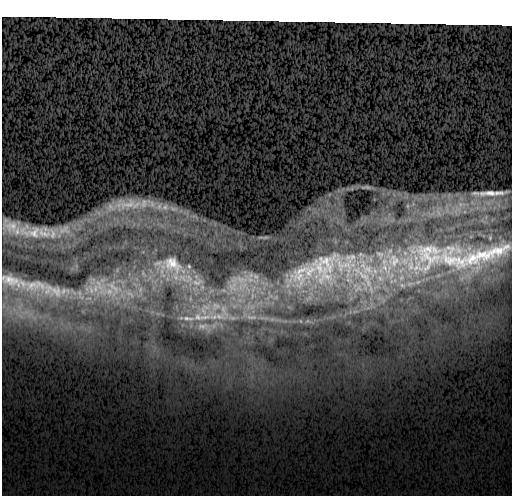
Impression: choroidal neovascularization.